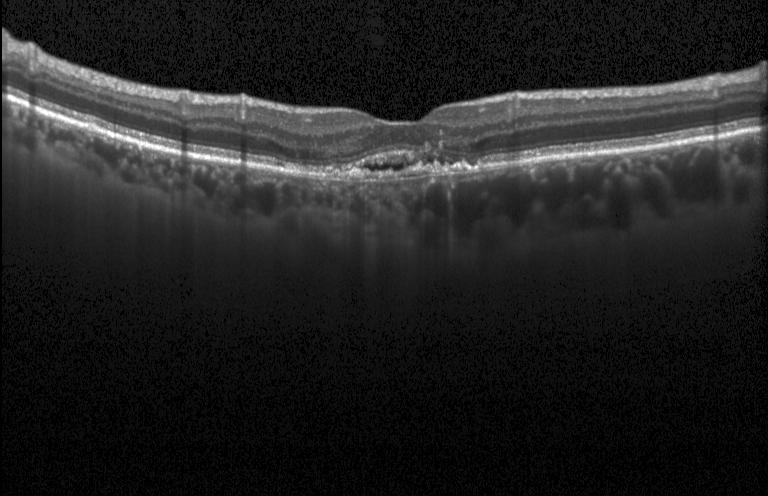 Spectral-domain OCT; Heidelberg Spectralis; OCT B-scan; through the macula — Assessment: a choroidal neovascular membrane.